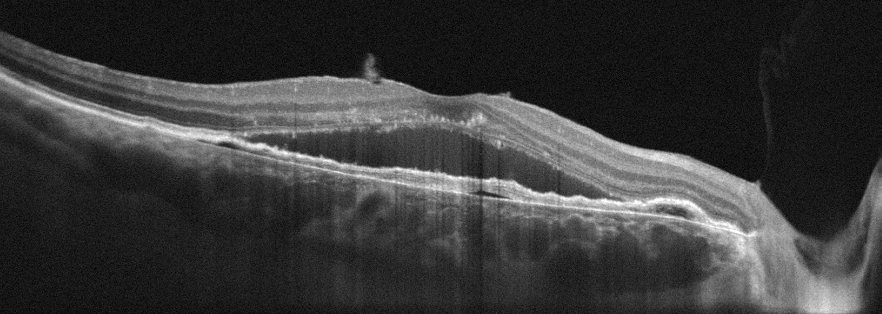
Instrument: Optovue Avanti RTVue XR · OD · optical coherence tomography B-scan · fovea-centered — Macular OCT: AMD.